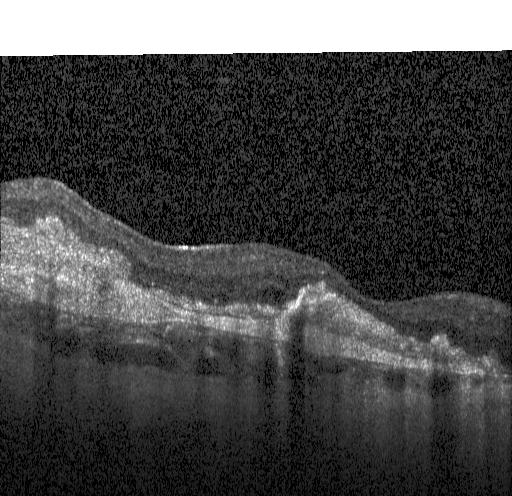
Retinal OCT cross-section. Impression: choroidal neovascularization (CNV).